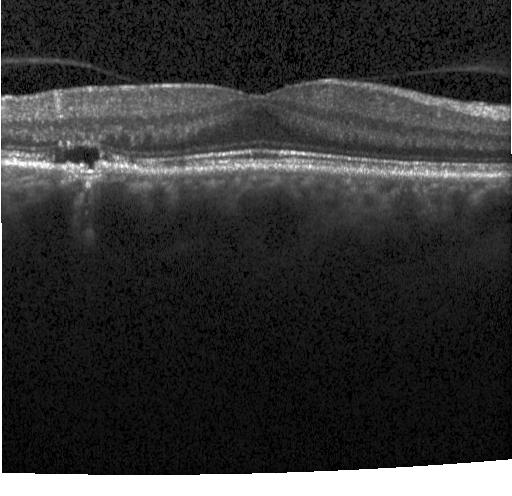

Retinal OCT B-scan — Assessment: a choroidal neovascular membrane.